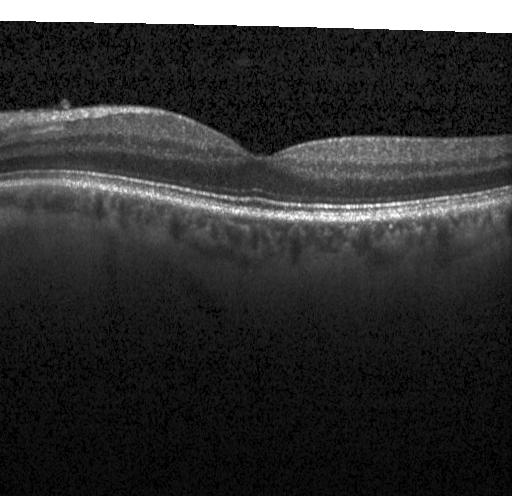

Optical coherence tomography B-scan
No CNV, no DME, and no drusen.